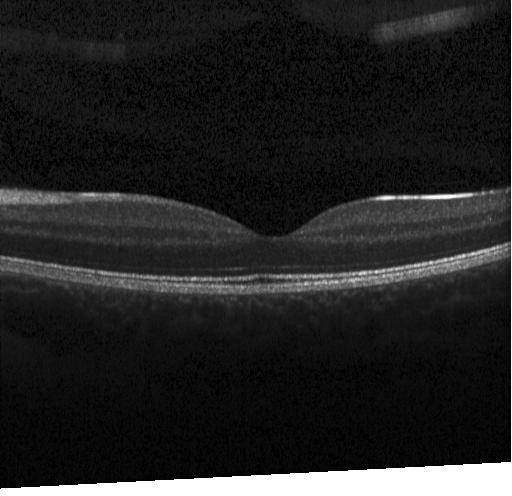

OCT B-scan showing no choroidal neovascularization, diabetic macular edema, or drusen.